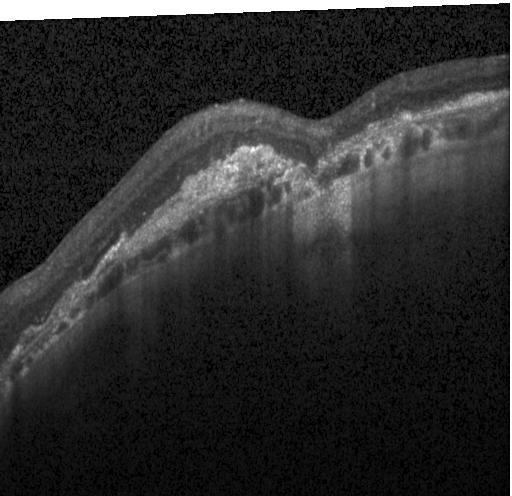 Optical coherence tomography scan, instrument: Heidelberg Spectralis, spectral-domain optical coherence tomography — A choroidal neovascular membrane.